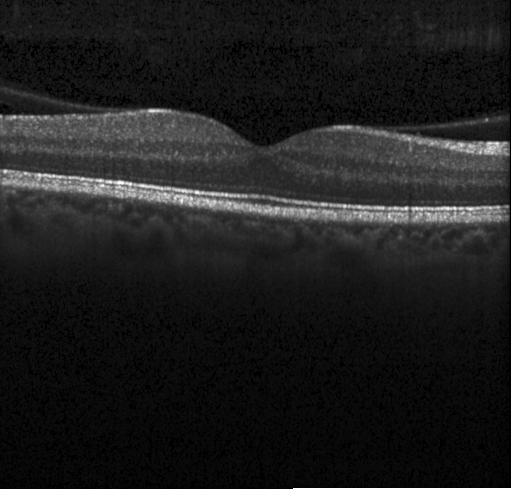
Retinal OCT cross-section — Diagnosis: no choroidal neovascularization, no diabetic macular edema, and no drusen.